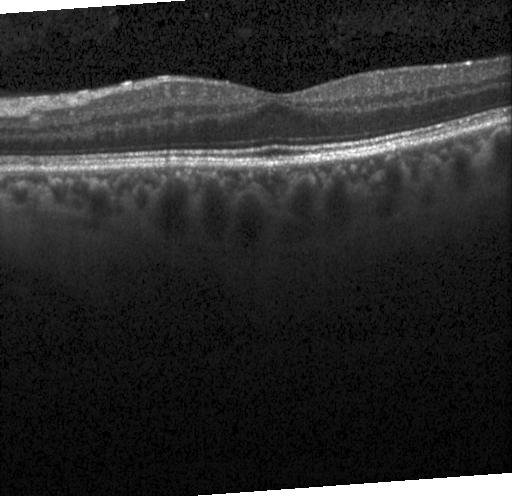

OCT B-scan
The scan shows no evidence of CNV, DME, or drusen.